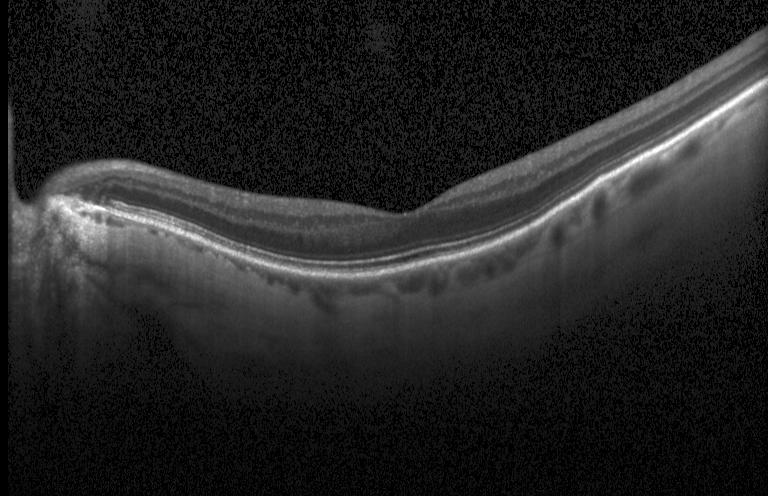

Horizontal scan through the fovea, OCT line scan.
Impression: no evidence of CNV, DME, or drusen.